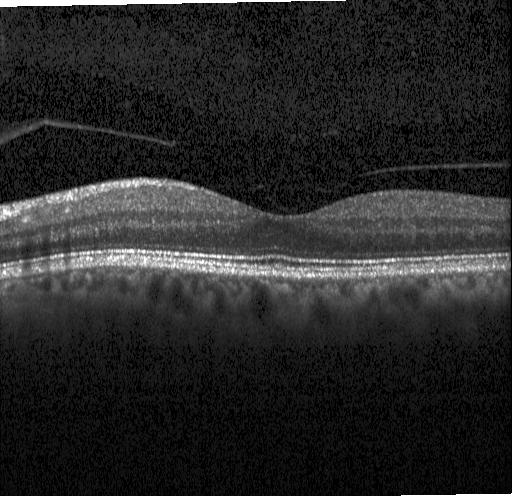

Optical coherence tomography scan. Spectral-domain optical coherence tomography.
Finding: no choroidal neovascularization, diabetic macular edema, or drusen.